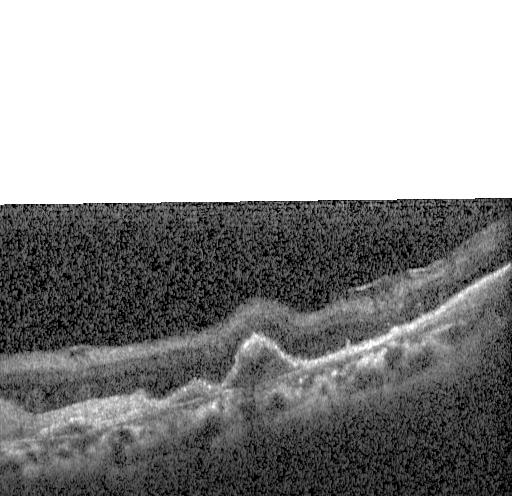
Spectral-domain optical coherence tomography, horizontal scan through the fovea, retinal OCT cross-section, Heidelberg Spectralis.
The scan shows a choroidal neovascular membrane.